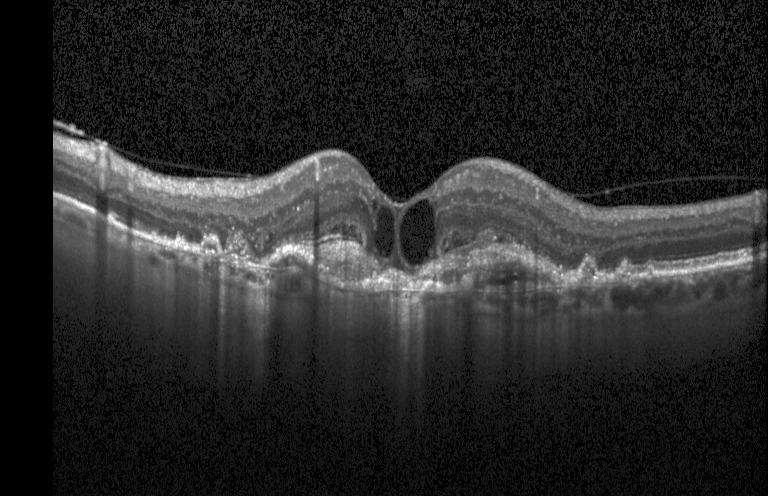

A choroidal neovascular membrane.